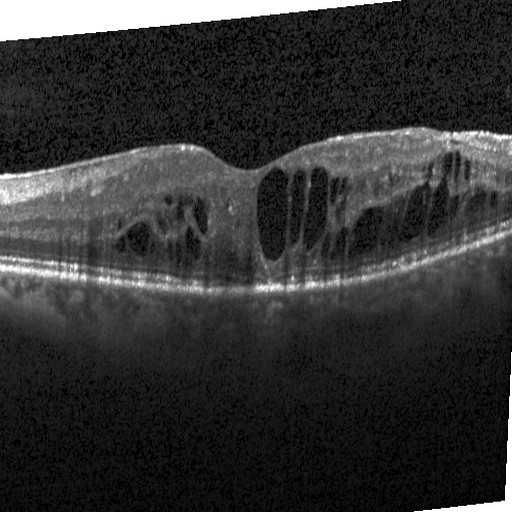

Retinal OCT cross-section — OCT finding: diabetic macular edema (DME).